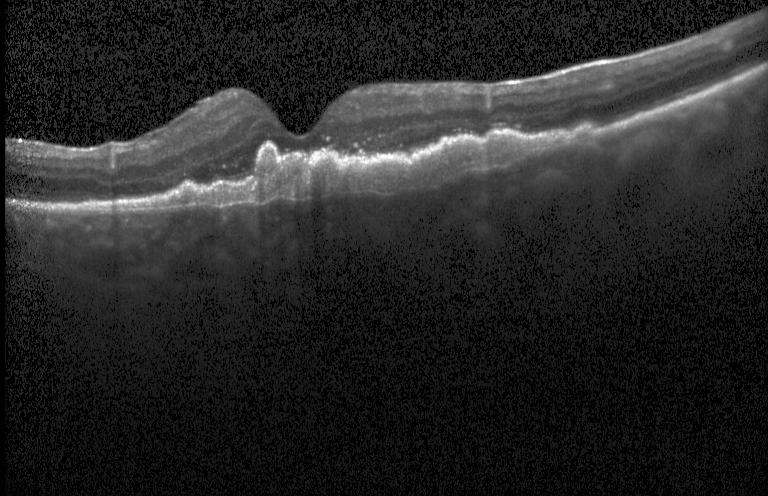

Diagnosis: CNV.